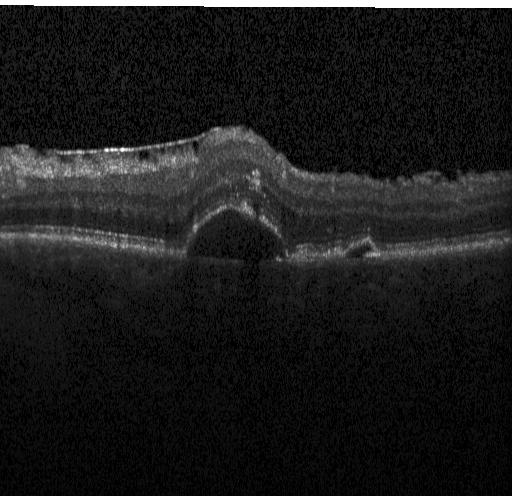
OCT line scan
Assessment: a choroidal neovascular membrane.